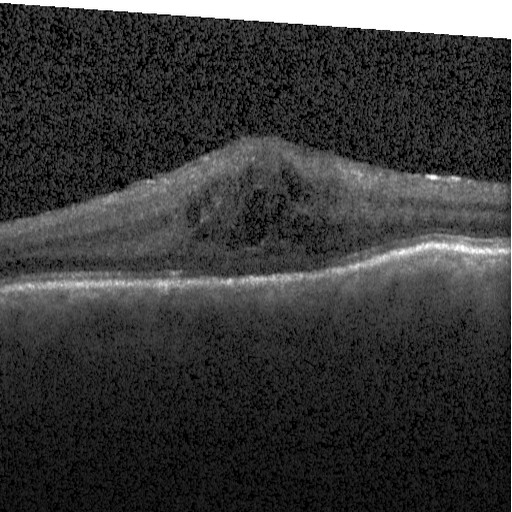 OCT scan showing DME.